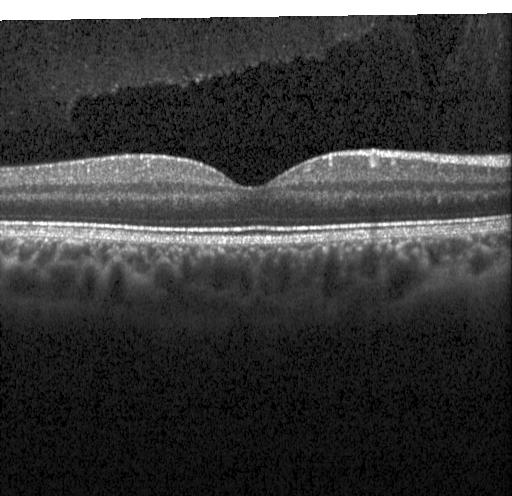
Dx: no choroidal neovascularization, no diabetic macular edema, and no drusen.